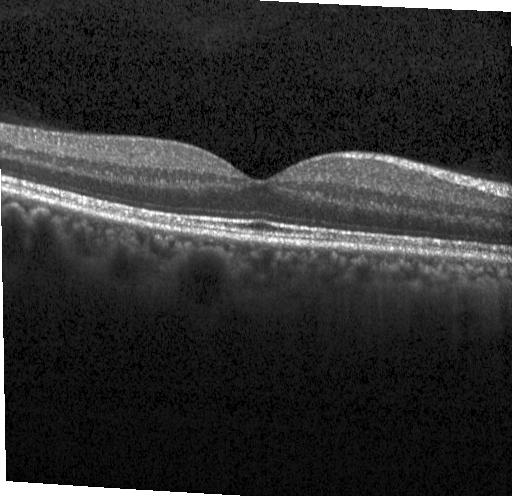
Neither choroidal neovascularization, diabetic macular edema, nor drusen.